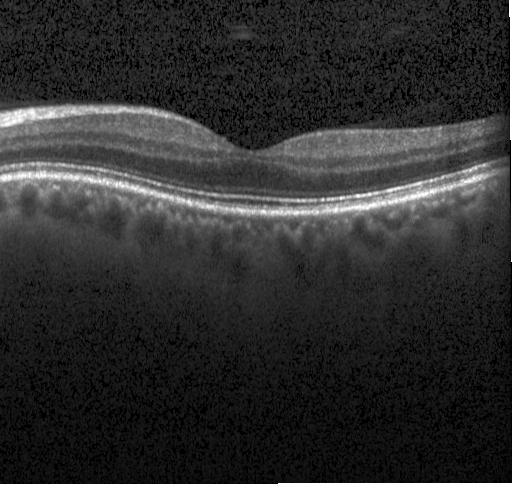

Optical coherence tomography B-scan.
This B-scan demonstrates no evidence of CNV, DME, or drusen.